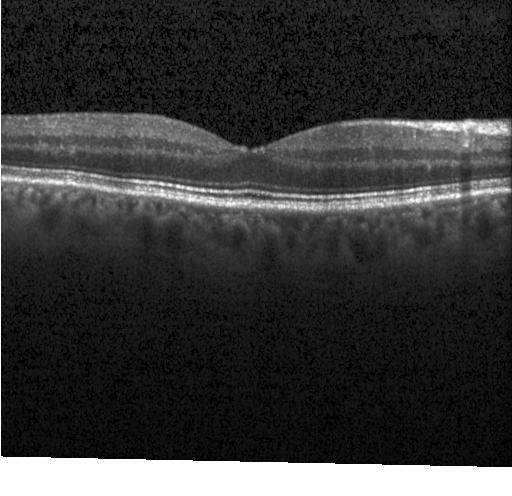 Optical coherence tomography scan; spectral-domain optical coherence tomography
Diagnosis: no CNV, DME, or drusen.